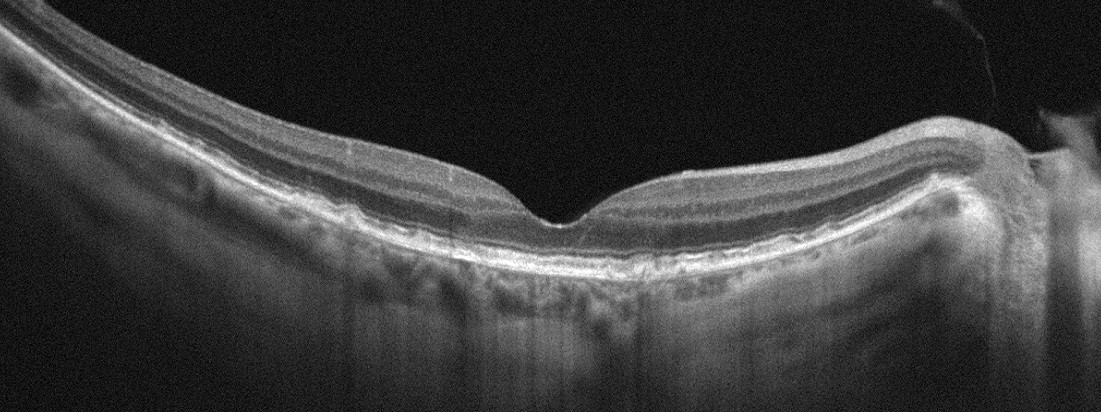
Retinal OCT cross-section
This B-scan demonstrates AMD.